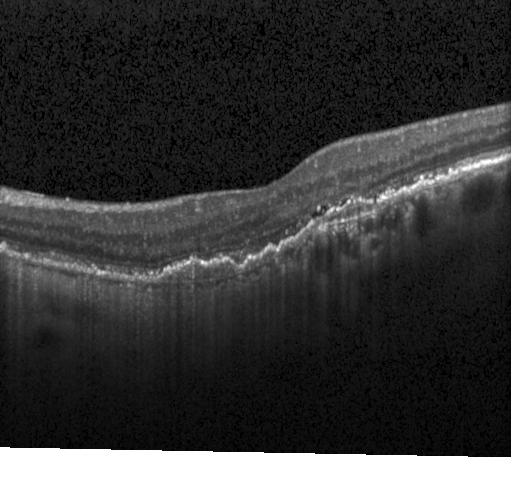

Diagnosis: a choroidal neovascular membrane.